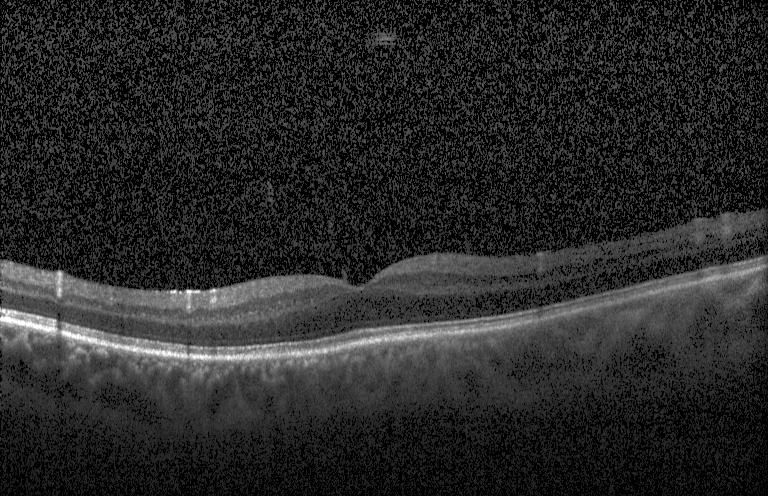 SD-OCT. Optical coherence tomography B-scan. Instrument: Heidelberg Spectralis. Horizontal scan through the fovea
Assessment: neither choroidal neovascularization, diabetic macular edema, nor drusen.